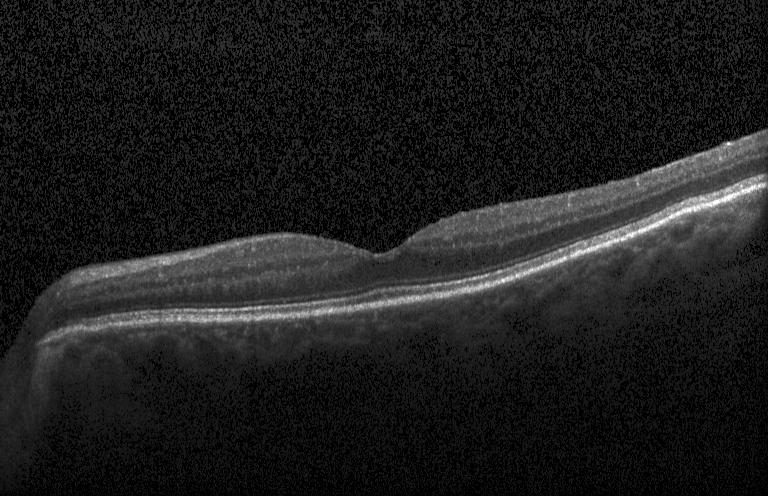

Spectral-domain OCT; instrument: Heidelberg Spectralis; retinal OCT cross-section; horizontal scan through the fovea. Macular OCT: no choroidal neovascularization, no diabetic macular edema, and no drusen.